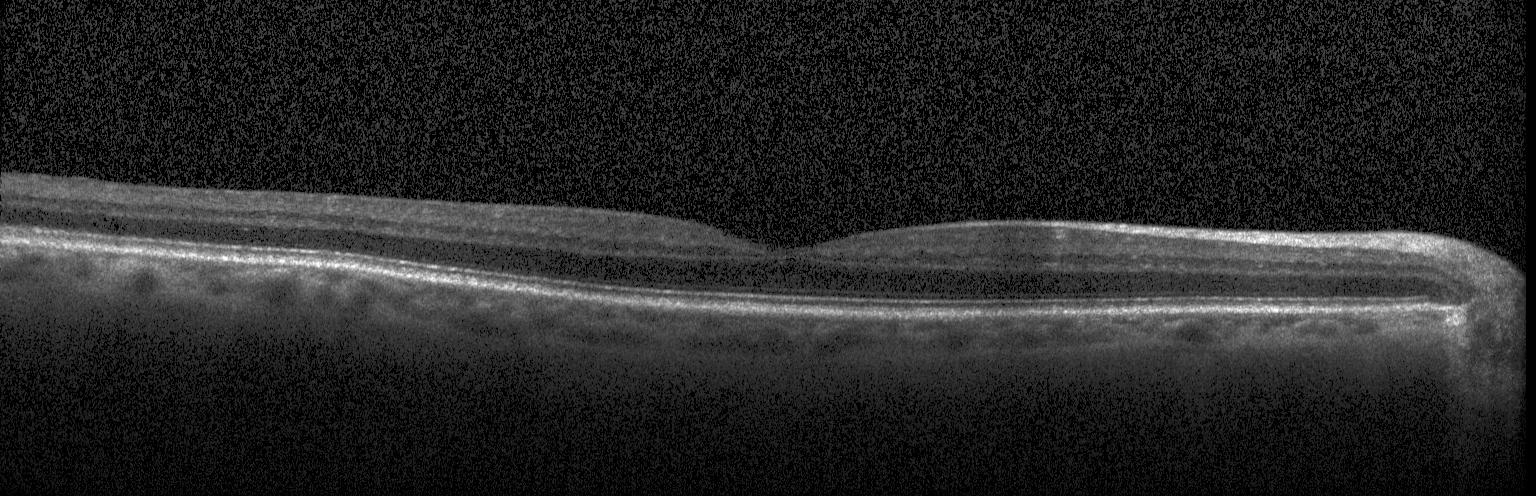

No CNV, no DME, and no drusen.